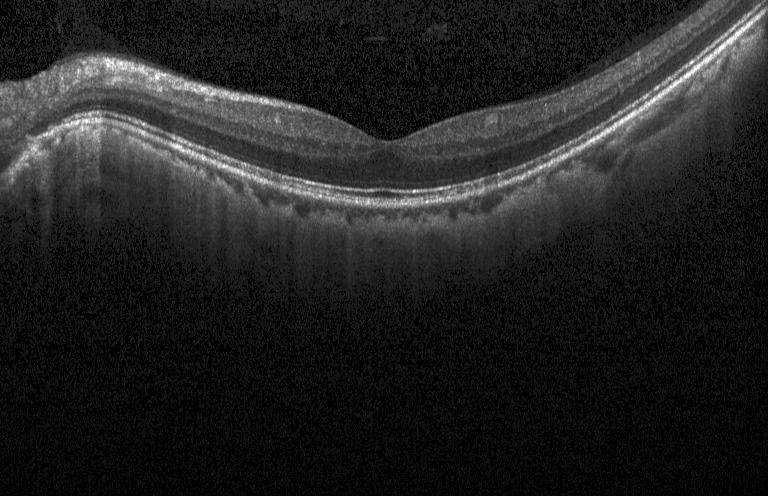
Diagnosis: neither CNV, DME, nor drusen.